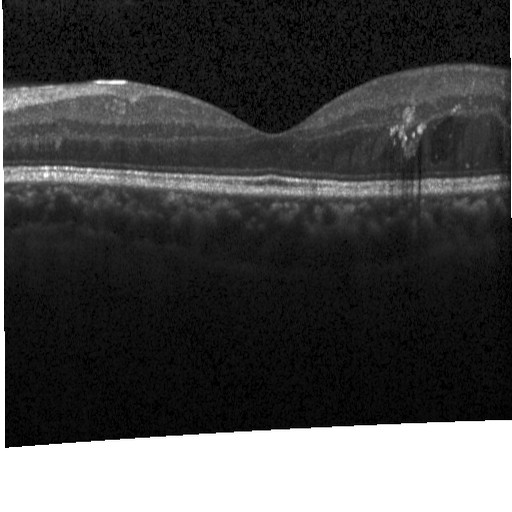
Optical coherence tomography scan
Diabetic macular edema.